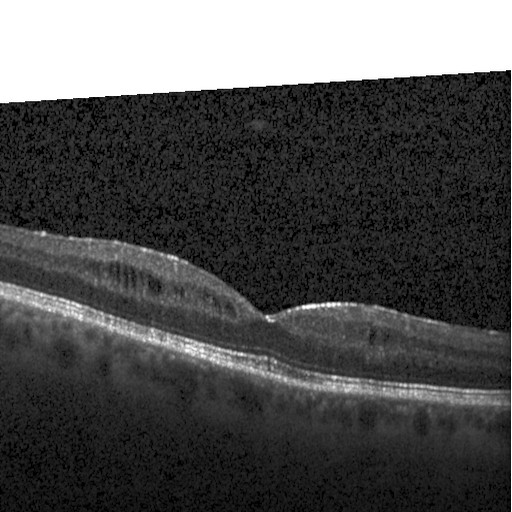 Impression: diabetic macular edema (DME).